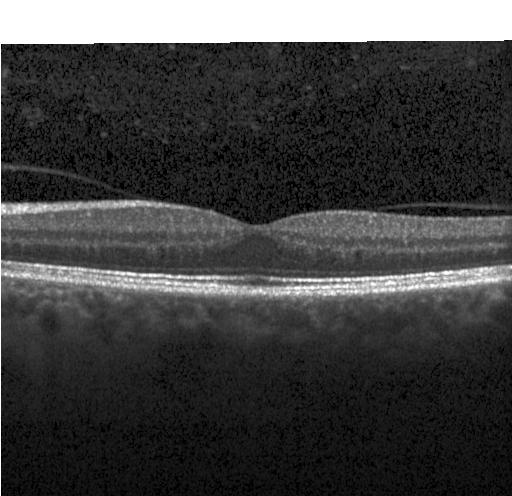

Through the macula · optical coherence tomography B-scan
No evidence of choroidal neovascularization, diabetic macular edema, or drusen.